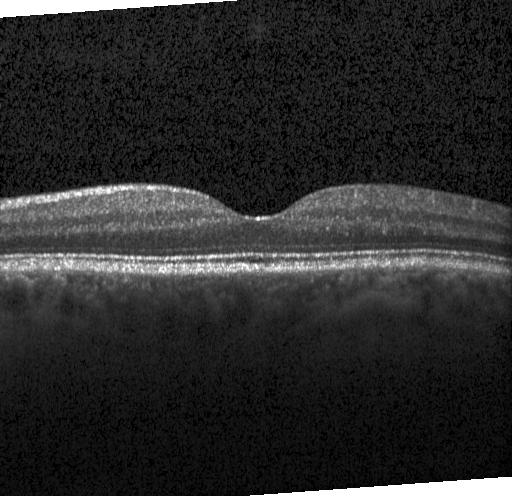

Centered on the fovea · Heidelberg Spectralis · optical coherence tomography scan · spectral-domain optical coherence tomography. Finding: neither choroidal neovascularization, diabetic macular edema, nor drusen.